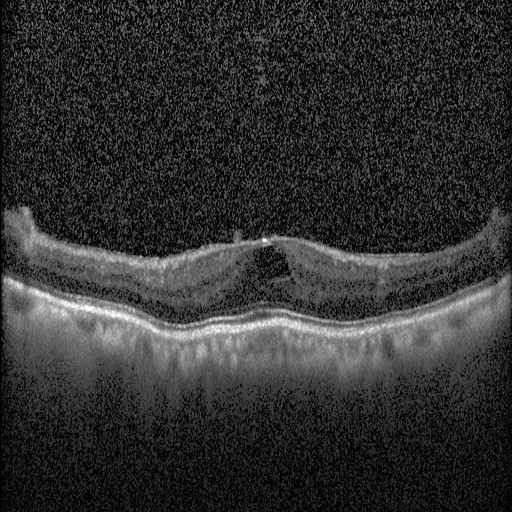

Retinal OCT cross-section · Heidelberg Spectralis. Impression: diabetic macular edema.